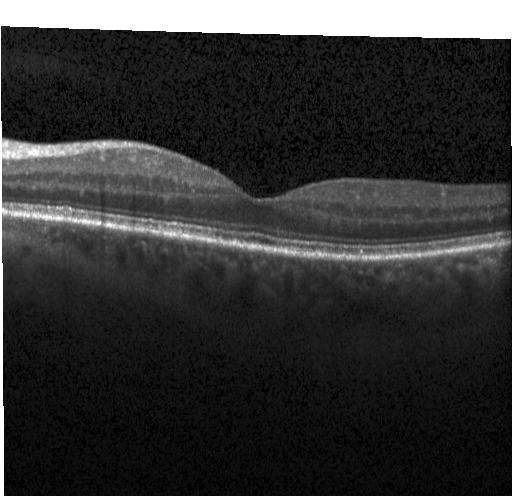
This B-scan demonstrates no evidence of CNV, DME, or drusen.